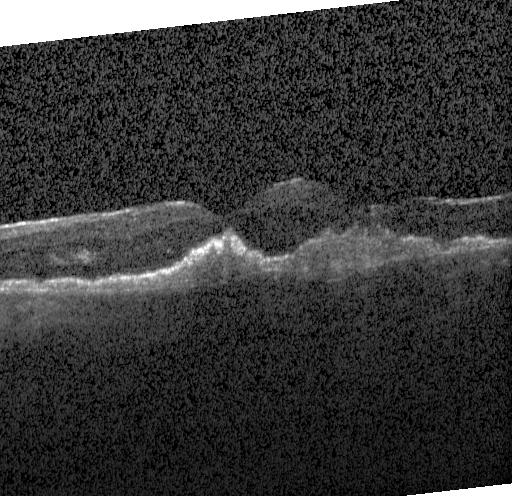

Diagnosis: a choroidal neovascular membrane.